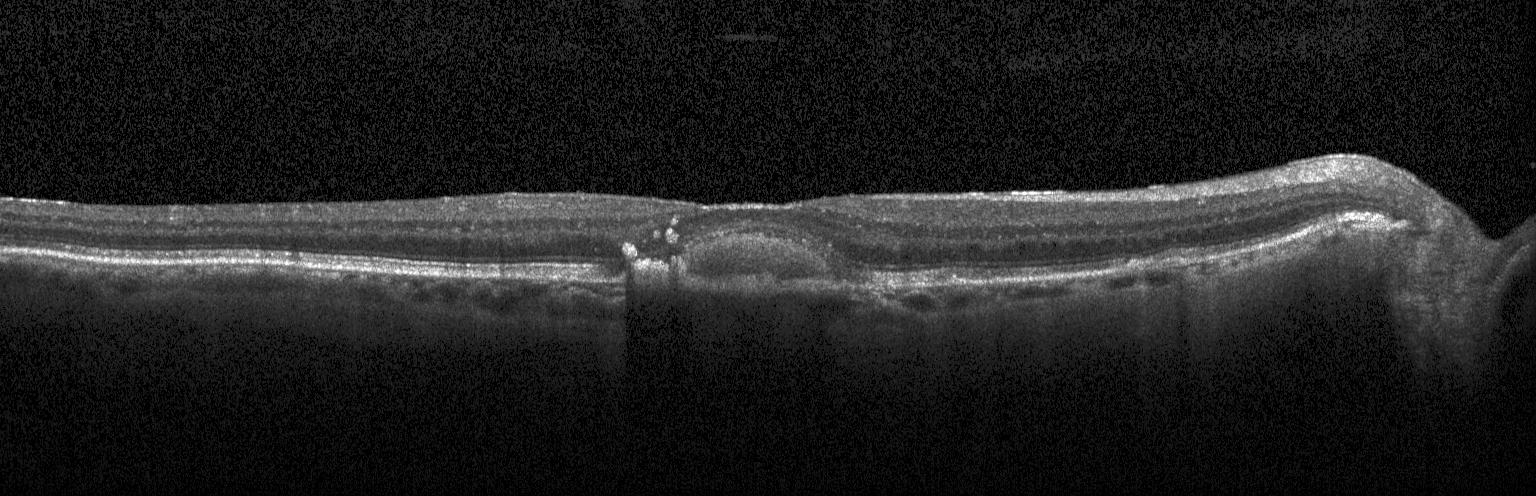 OCT scan showing CNV.